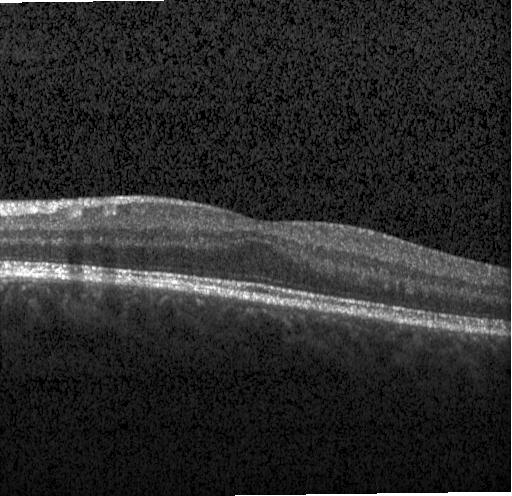
Instrument: Heidelberg Spectralis, retinal OCT B-scan, spectral-domain optical coherence tomography
Impression: no choroidal neovascularization, no diabetic macular edema, and no drusen.